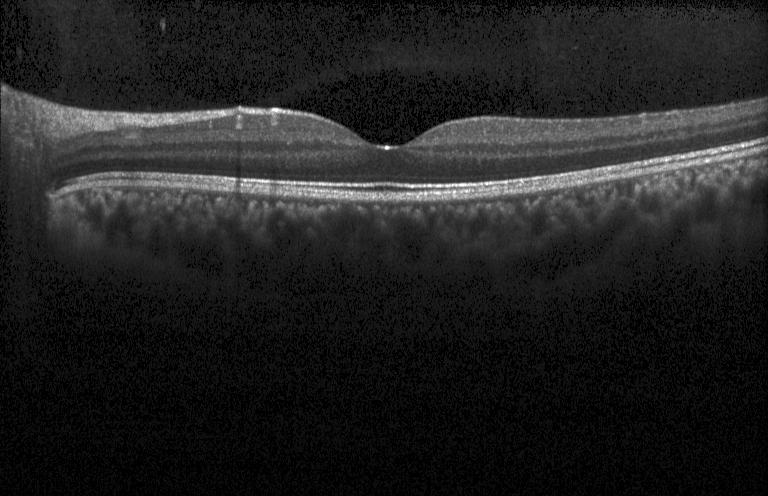 Optical coherence tomography B-scan · horizontal scan through the fovea.
Diagnosis: no choroidal neovascularization, diabetic macular edema, or drusen.